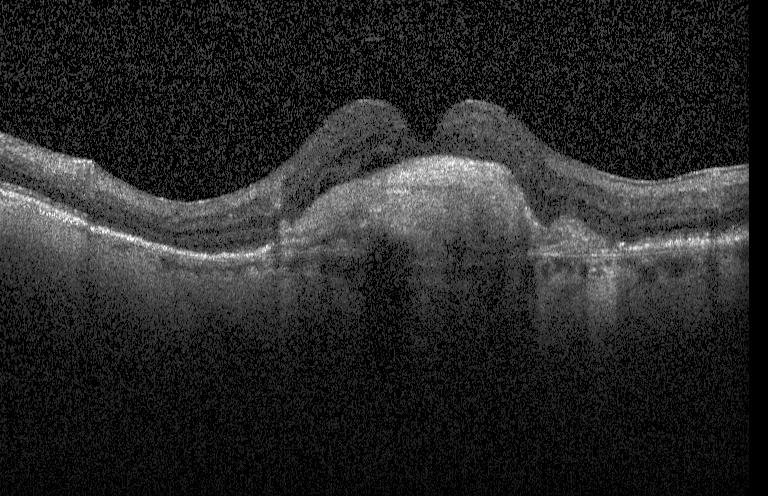 Retinal OCT cross-section, spectral-domain optical coherence tomography, instrument: Heidelberg Spectralis, centered on the fovea
Finding: choroidal neovascularization.